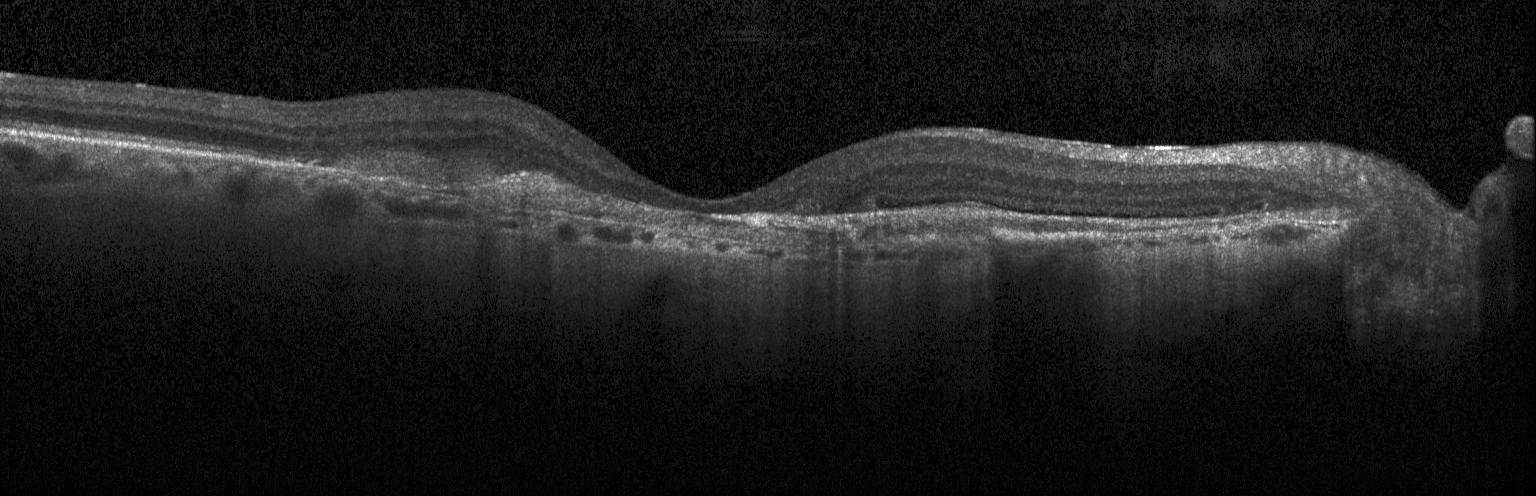
Optical coherence tomography B-scan; Heidelberg Spectralis OCT system; SD-OCT; fovea-centered — Macular OCT: a choroidal neovascular membrane.